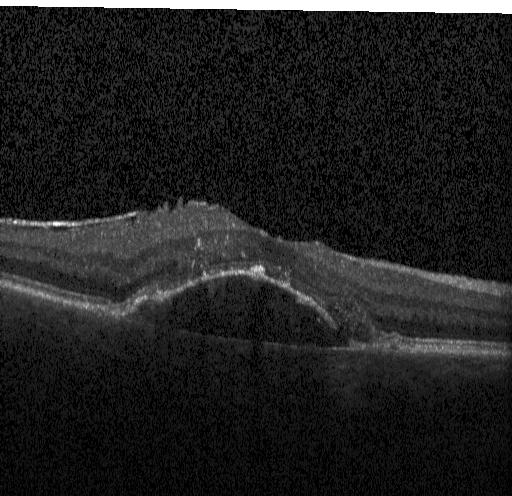
Diagnosis: choroidal neovascularization.